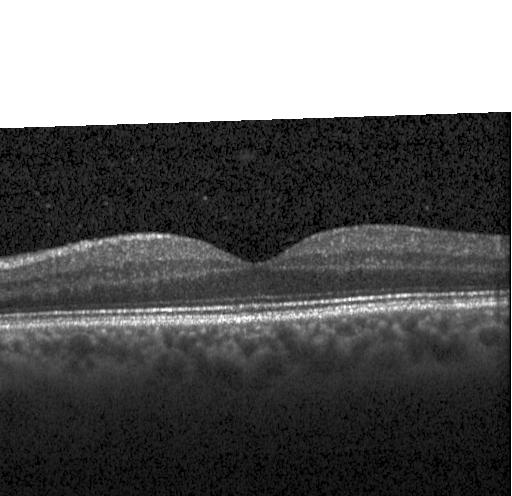

SD-OCT · instrument: Heidelberg Spectralis · retinal OCT cross-section
Finding: no choroidal neovascularization, diabetic macular edema, or drusen.